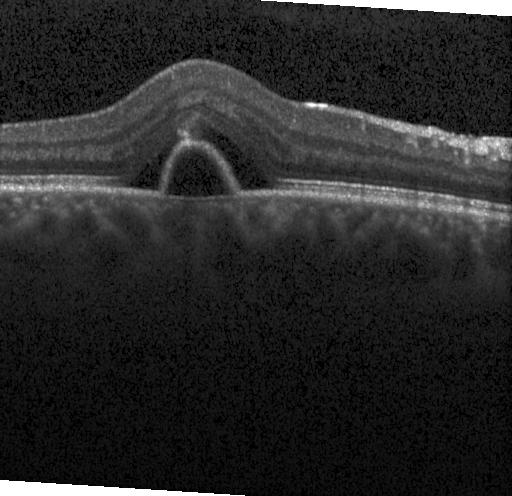

Retinal OCT cross-section. The scan shows a choroidal neovascular membrane.